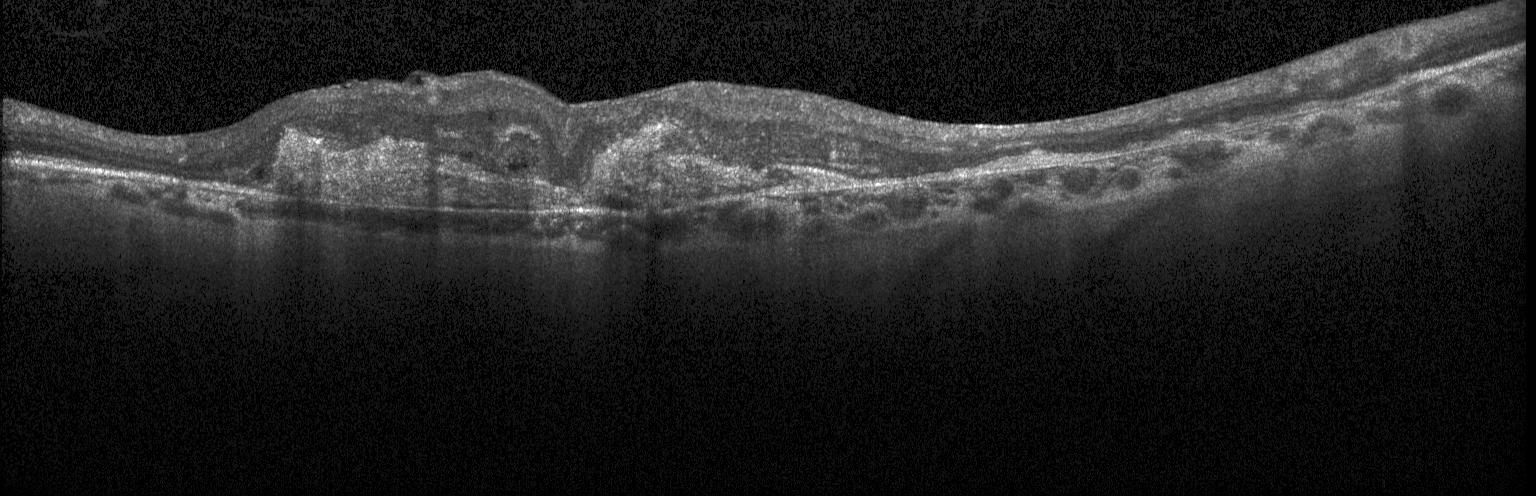 Macular OCT: a choroidal neovascular membrane.